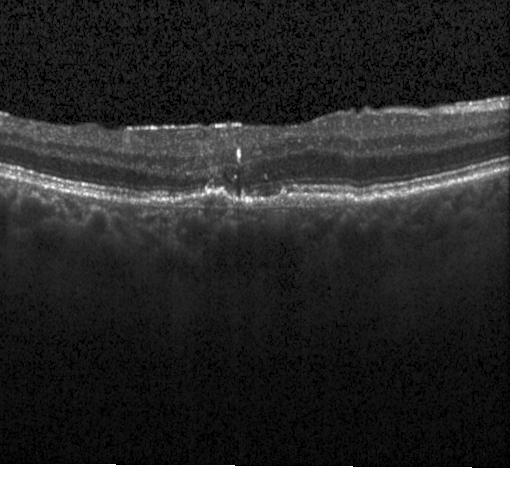 Retinal OCT B-scan; spectral-domain OCT.
The scan shows a choroidal neovascular membrane.